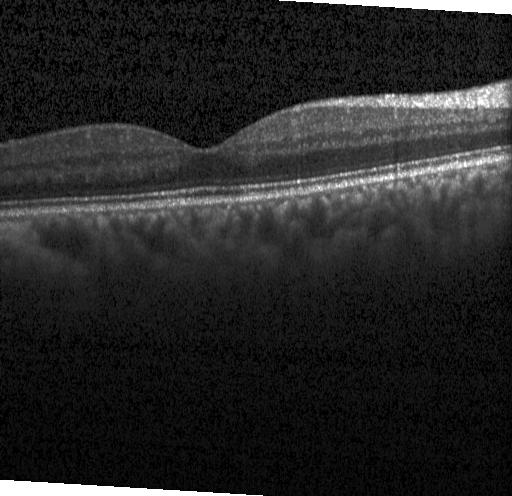
Retinal OCT cross-section showing no choroidal neovascularization, no diabetic macular edema, and no drusen.